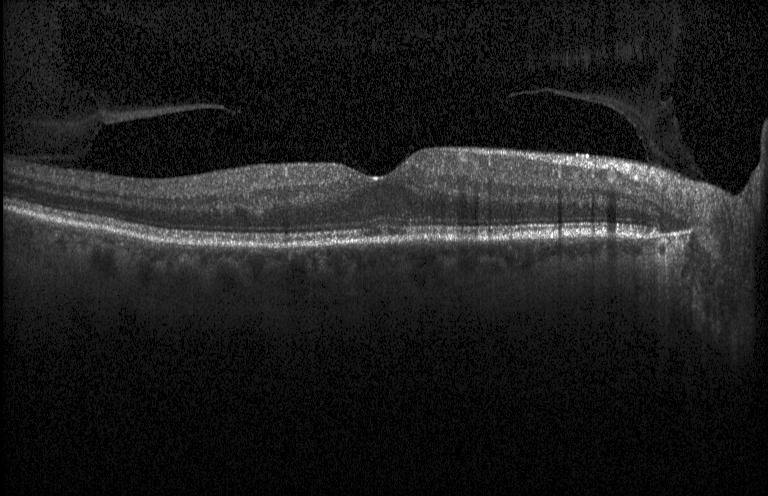 Retinal OCT cross-section showing neither CNV, DME, nor drusen.